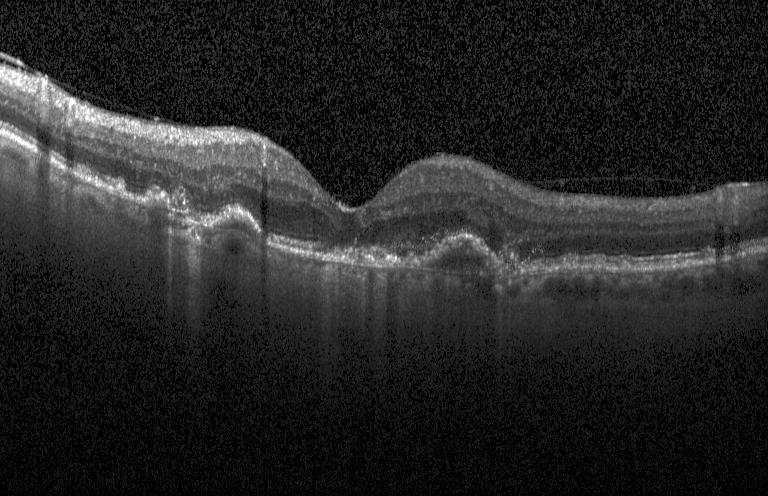 Impression: CNV.